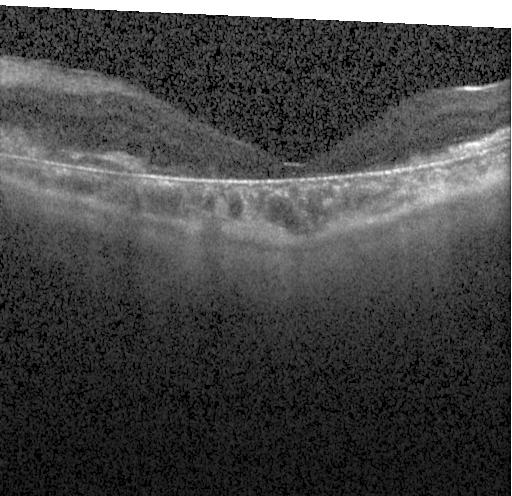
Impression: choroidal neovascularization (CNV).